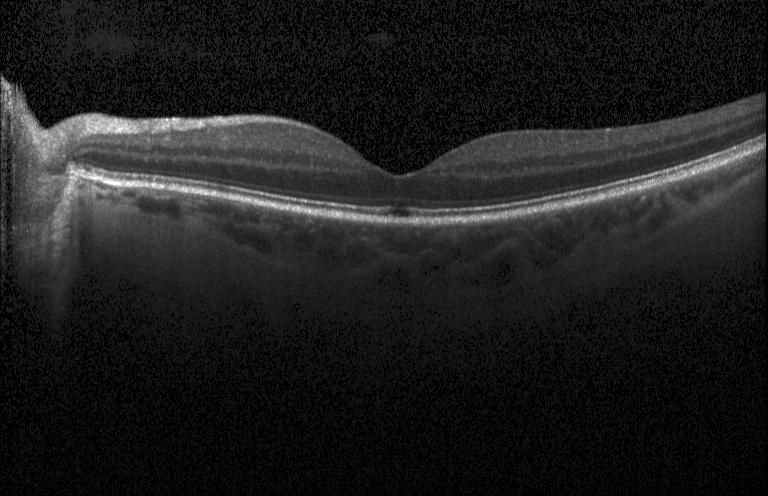
Spectral-domain OCT, fovea-centered, OCT B-scan. The scan shows no evidence of choroidal neovascularization, diabetic macular edema, or drusen.